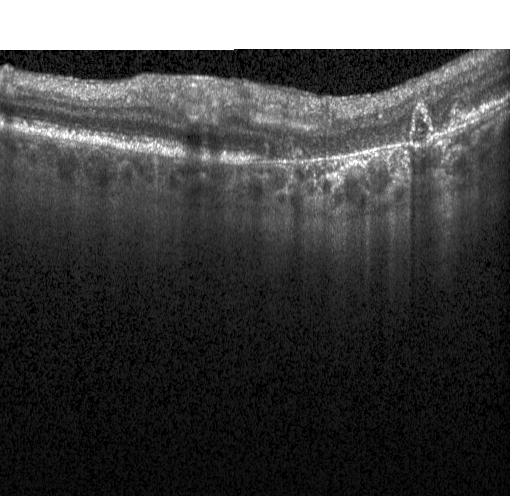 OCT scan showing choroidal neovascularization.